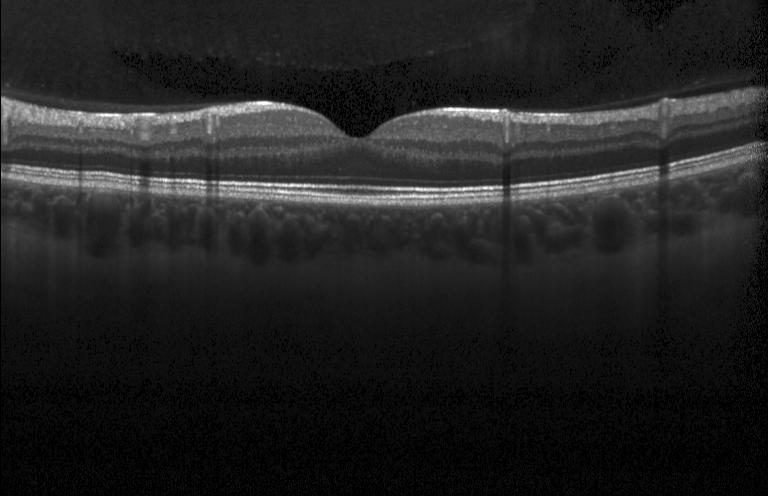 Spectral-domain OCT, macular scan, instrument: Heidelberg Spectralis, retinal OCT cross-section
Diagnosis: no CNV, DME, or drusen.